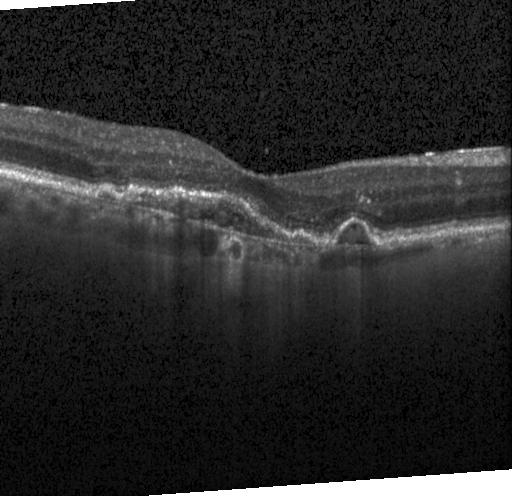
SD-OCT · instrument: Heidelberg Spectralis · optical coherence tomography B-scan — Impression: choroidal neovascularization (CNV).